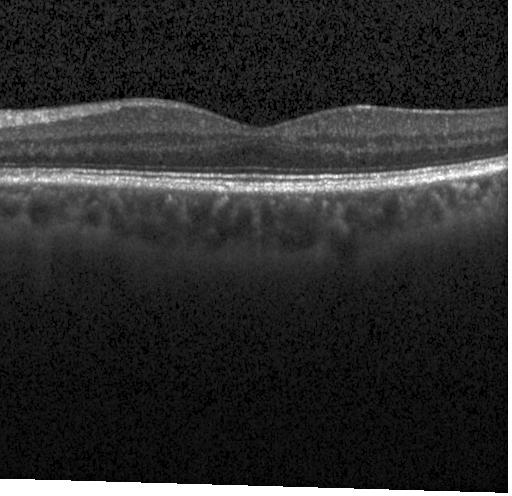

Instrument: Heidelberg Spectralis · spectral-domain optical coherence tomography · OCT B-scan. This B-scan demonstrates no choroidal neovascularization, no diabetic macular edema, and no drusen.